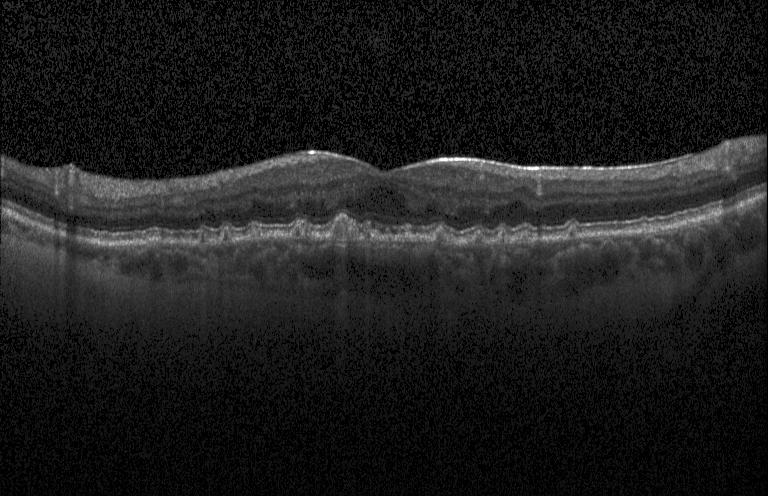 Heidelberg Spectralis, retinal OCT B-scan, through the macula, SD-OCT. Multiple drusen.